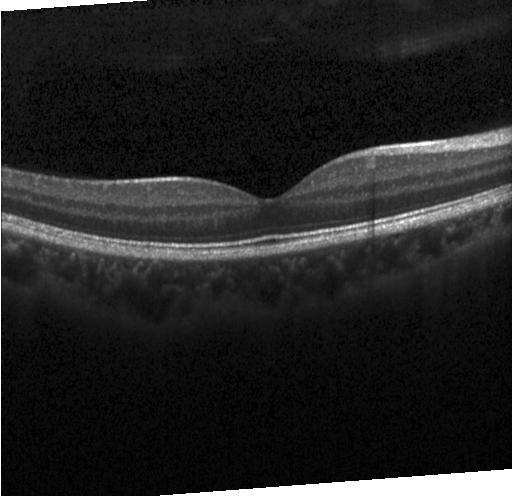 OCT scan showing neither choroidal neovascularization, diabetic macular edema, nor drusen.